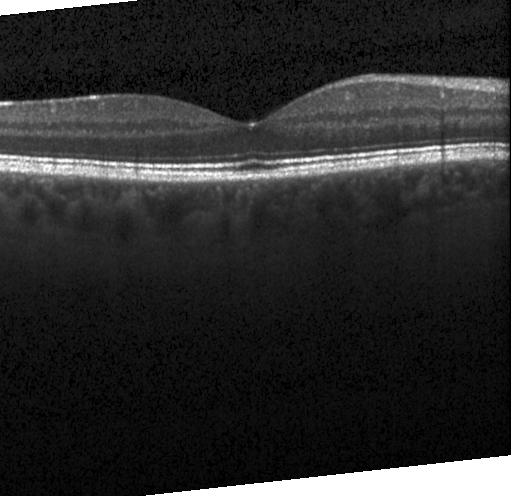 Optical coherence tomography B-scan. SD-OCT. Macular scan — OCT finding: no evidence of choroidal neovascularization, diabetic macular edema, or drusen.